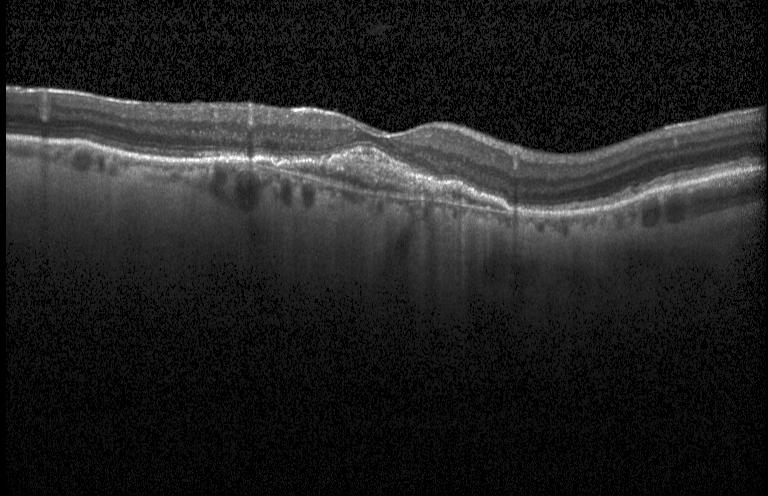 Optical coherence tomography B-scan. The scan shows CNV.